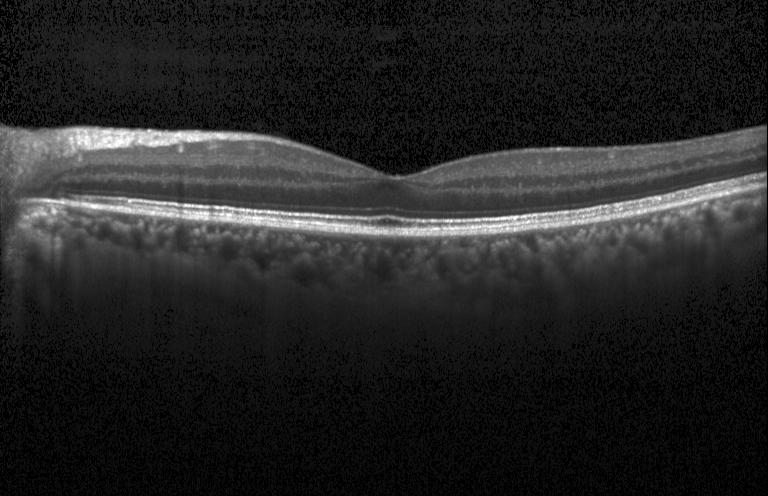

This B-scan demonstrates no choroidal neovascularization, diabetic macular edema, or drusen.